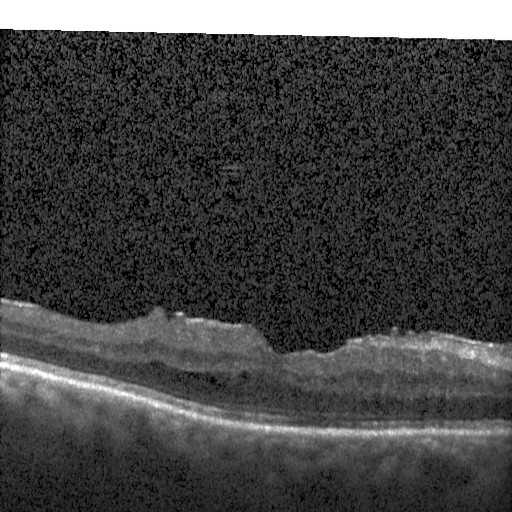

Retinal OCT cross-section · centered on the fovea. Impression: DME.